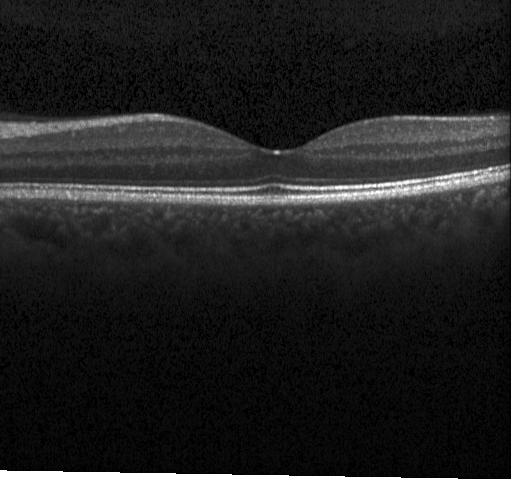 Fovea-centered · optical coherence tomography B-scan · spectral-domain OCT · acquired on a Heidelberg Spectralis — Dx: no choroidal neovascularization, diabetic macular edema, or drusen.